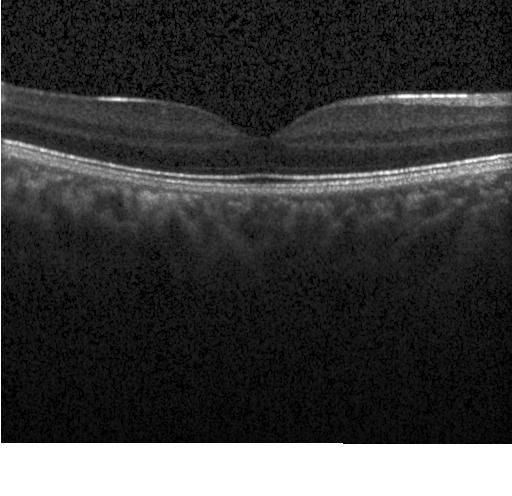
No choroidal neovascularization, diabetic macular edema, or drusen.